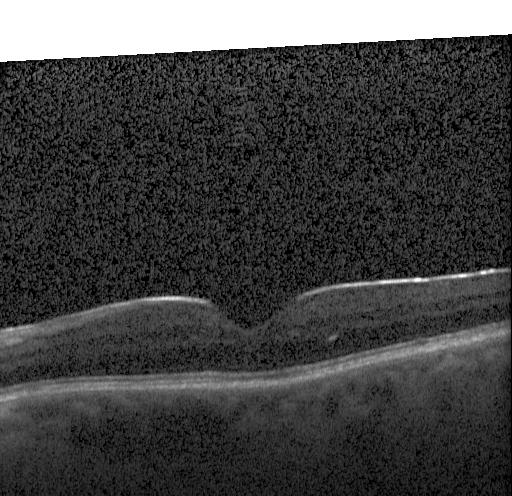
Instrument: Heidelberg Spectralis; OCT B-scan
No choroidal neovascularization, diabetic macular edema, or drusen.